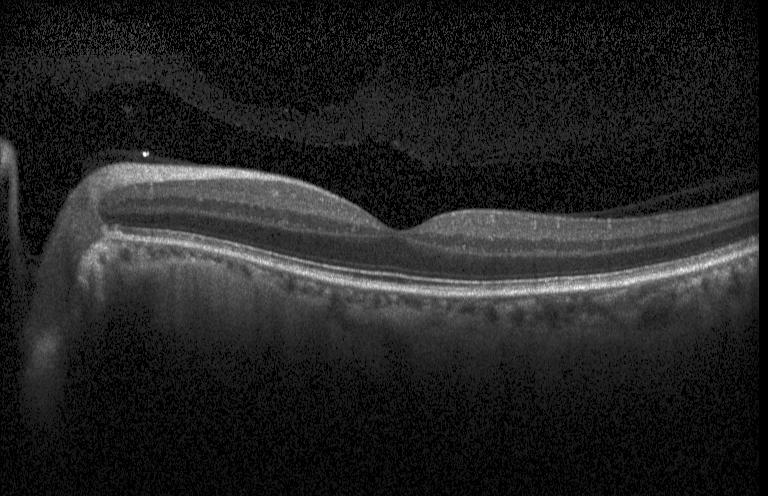
OCT line scan.
This B-scan demonstrates no evidence of choroidal neovascularization, diabetic macular edema, or drusen.